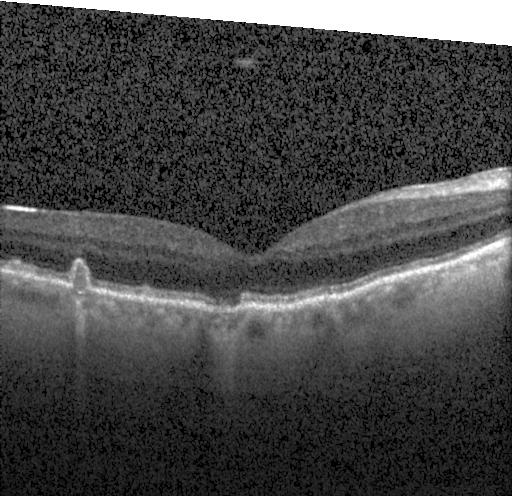
Diagnosis: sub-RPE drusenoid deposits.